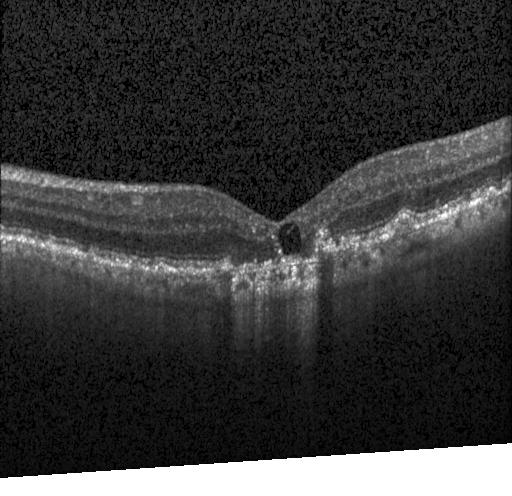
Retinal OCT B-scan.
Dx: a choroidal neovascular membrane.